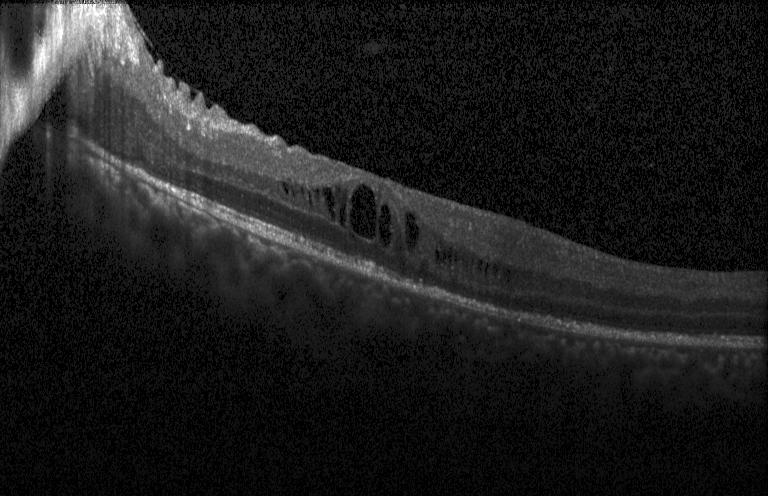 OCT B-scan.
This B-scan demonstrates diabetic macular edema (DME).